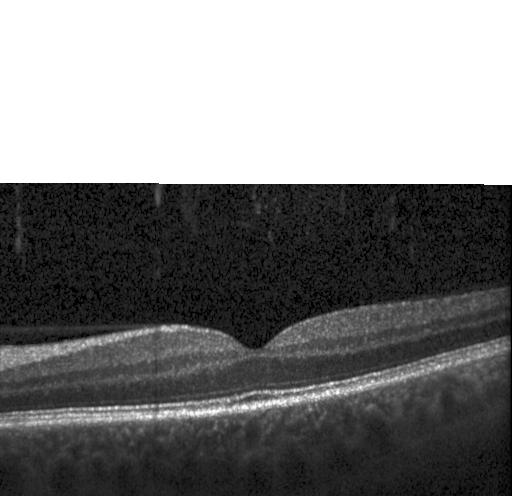
Optical coherence tomography B-scan — Diagnosis: no CNV, no DME, and no drusen.